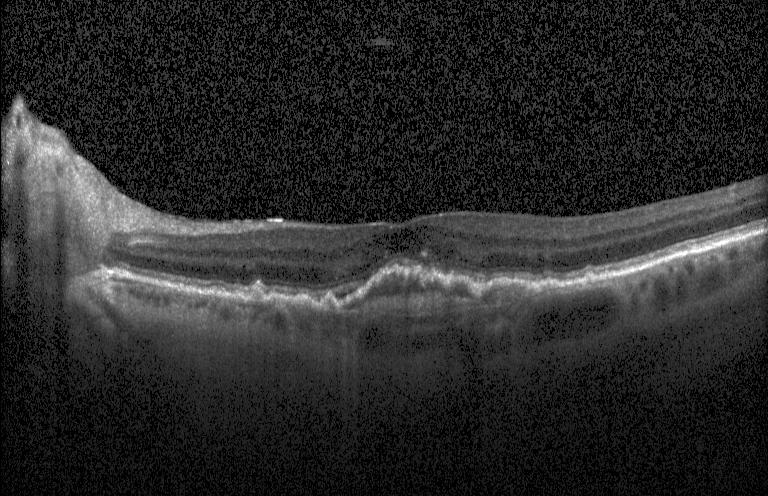
Optical coherence tomography B-scan. Heidelberg Spectralis OCT system. Horizontal scan through the fovea. Finding: a choroidal neovascular membrane.